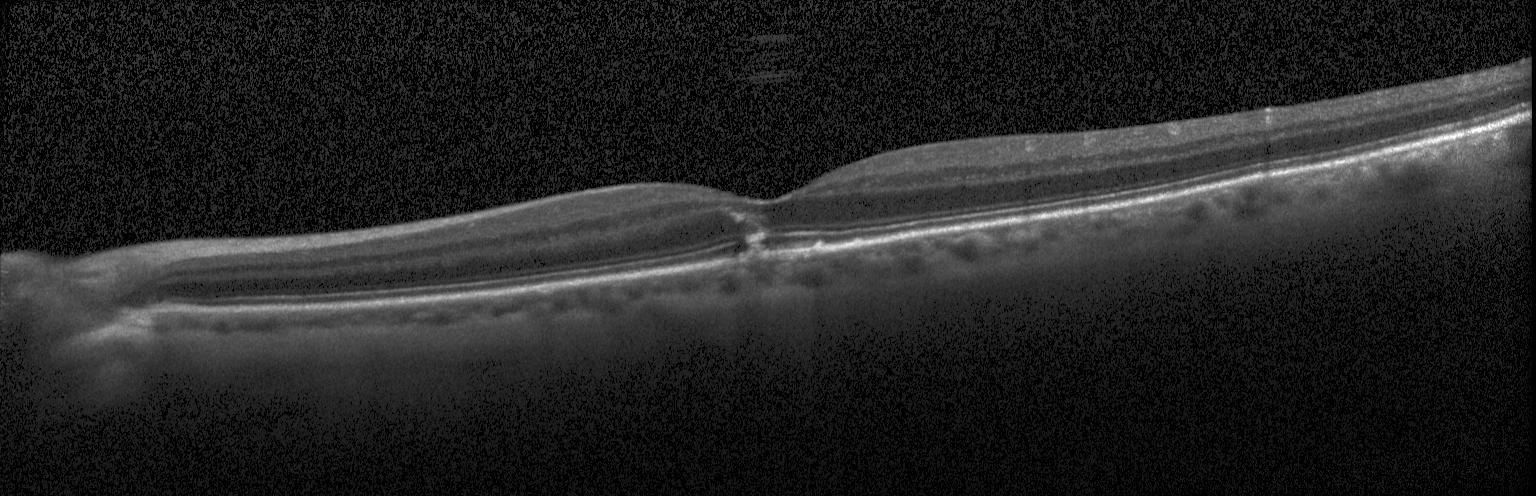
The scan shows a choroidal neovascular membrane.